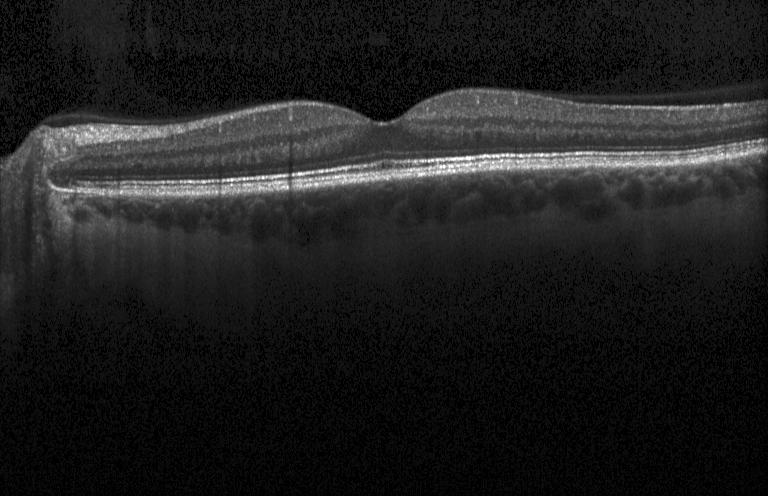

Spectral-domain optical coherence tomography. Through the macula. Retinal OCT B-scan
Impression: no choroidal neovascularization, diabetic macular edema, or drusen.